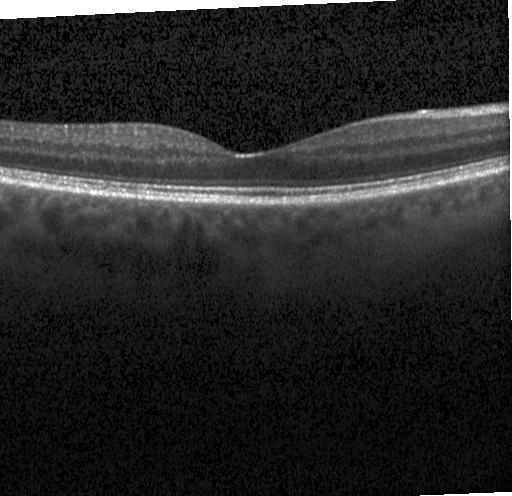

Macular scan. OCT line scan. Instrument: Heidelberg Spectralis. Macular OCT: no CNV, no DME, and no drusen.